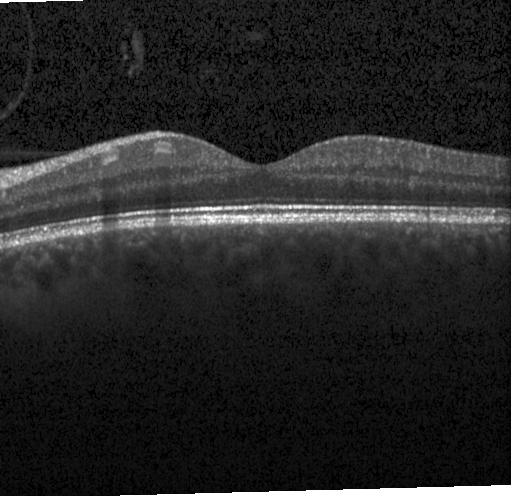

Retinal OCT cross-section. Spectral-domain OCT — Assessment: no evidence of choroidal neovascularization, diabetic macular edema, or drusen.